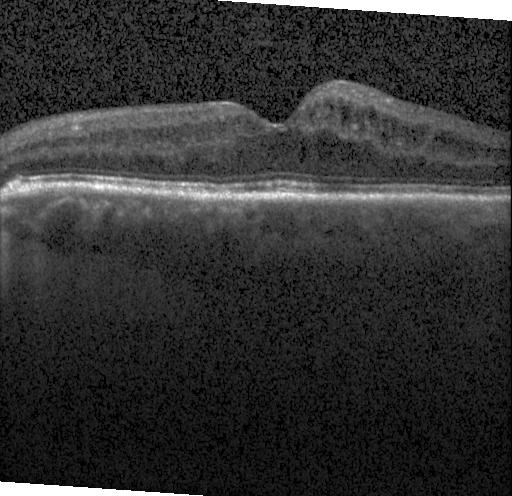
DME.